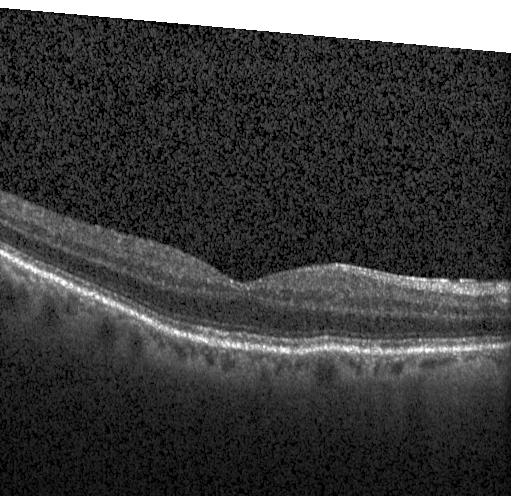

Finding: no CNV, no DME, and no drusen.